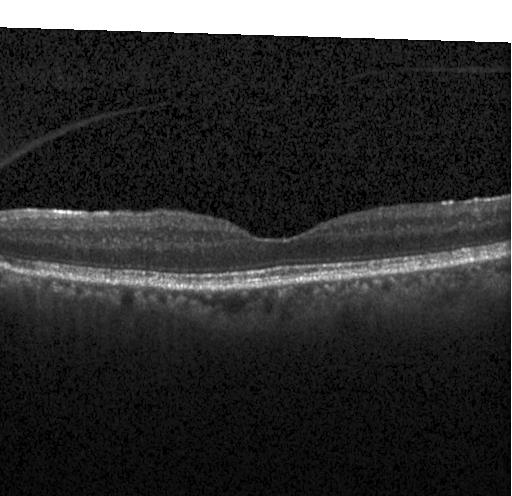
Heidelberg Spectralis OCT system, centered on the fovea, retinal OCT cross-section, spectral-domain OCT. Diagnosis: neither choroidal neovascularization, diabetic macular edema, nor drusen.